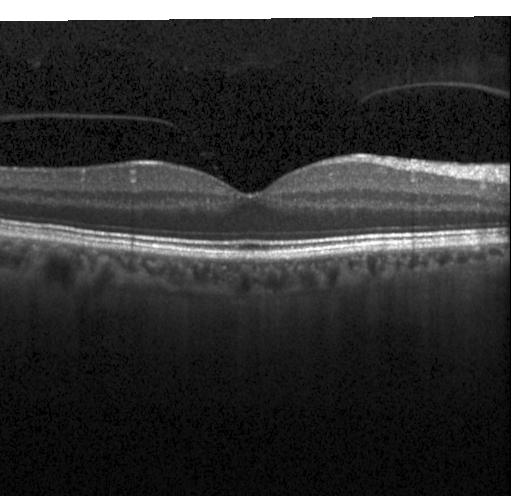

Optical coherence tomography B-scan. Fovea-centered. Spectral-domain optical coherence tomography.
Assessment: neither choroidal neovascularization, diabetic macular edema, nor drusen.